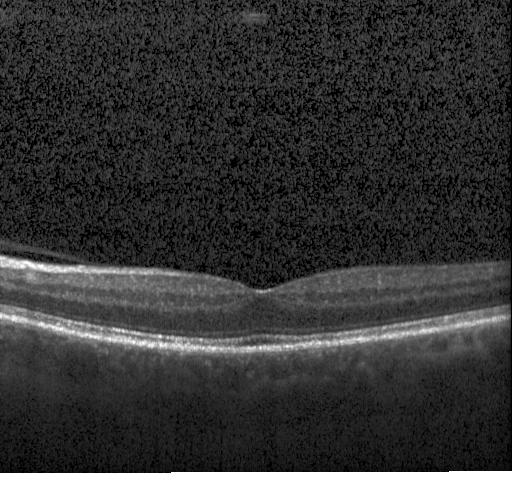

Optical coherence tomography scan, Heidelberg Spectralis OCT system — This B-scan demonstrates no evidence of choroidal neovascularization, diabetic macular edema, or drusen.